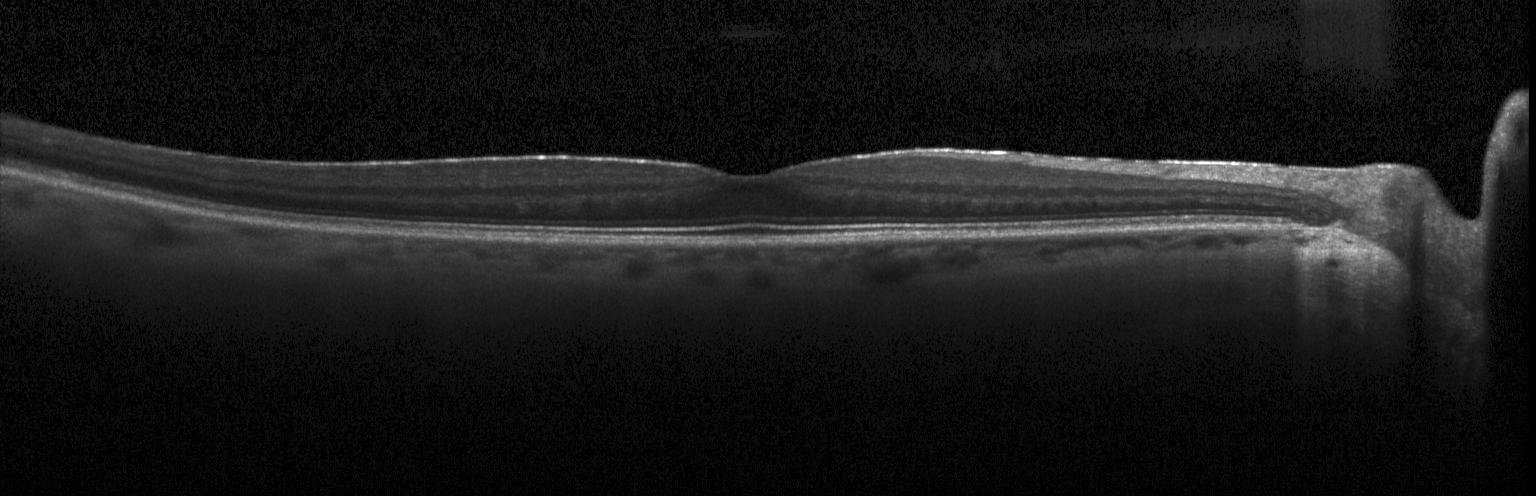 Impression: no choroidal neovascularization, diabetic macular edema, or drusen.